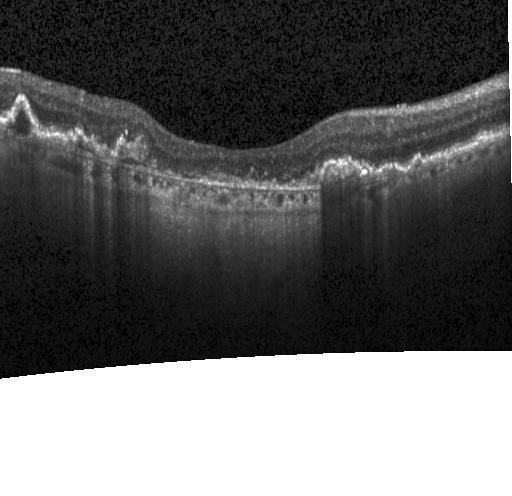 OCT line scan, spectral-domain optical coherence tomography
Impression: choroidal neovascularization (CNV).